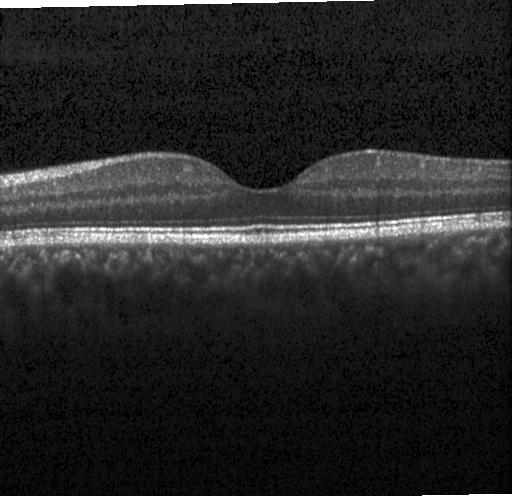

Optical coherence tomography scan.
Diagnosis: no evidence of choroidal neovascularization, diabetic macular edema, or drusen.